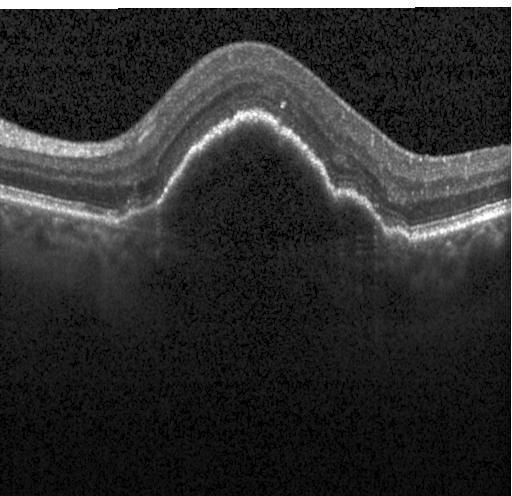
Horizontal scan through the fovea; spectral-domain optical coherence tomography; optical coherence tomography scan
CNV.